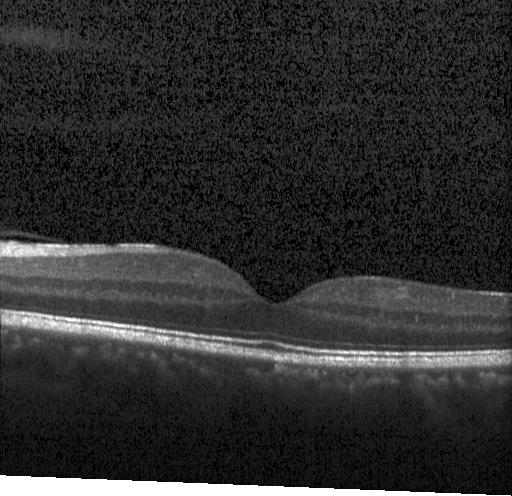

OCT B-scan. Centered on the fovea
Finding: no evidence of choroidal neovascularization, diabetic macular edema, or drusen.